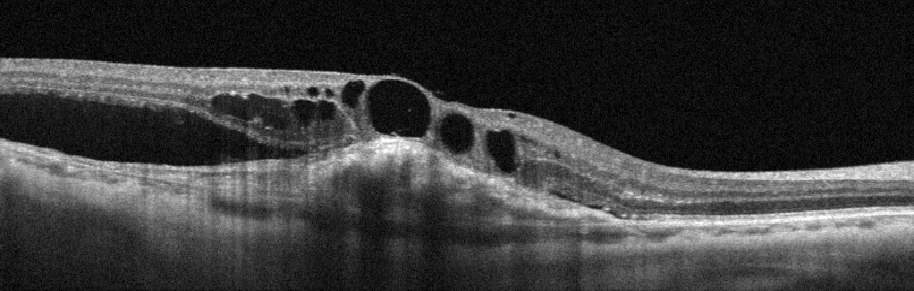
Optical coherence tomography scan. Right eye.
Impression: AMD.